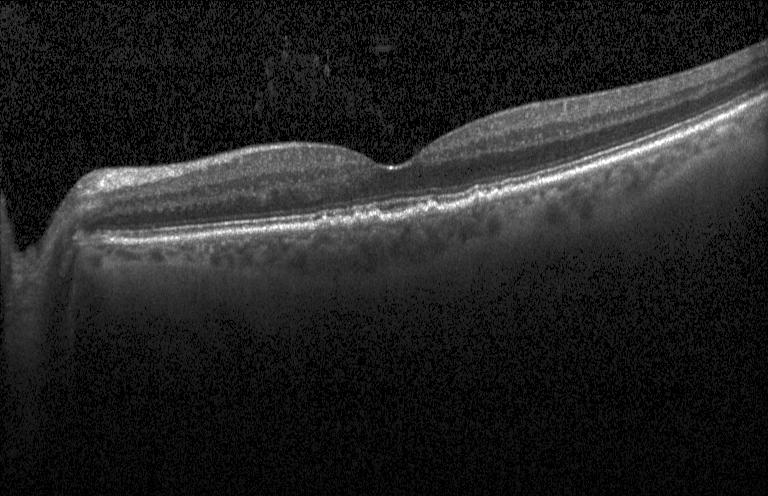

Optical coherence tomography B-scan.
Finding: drusen.